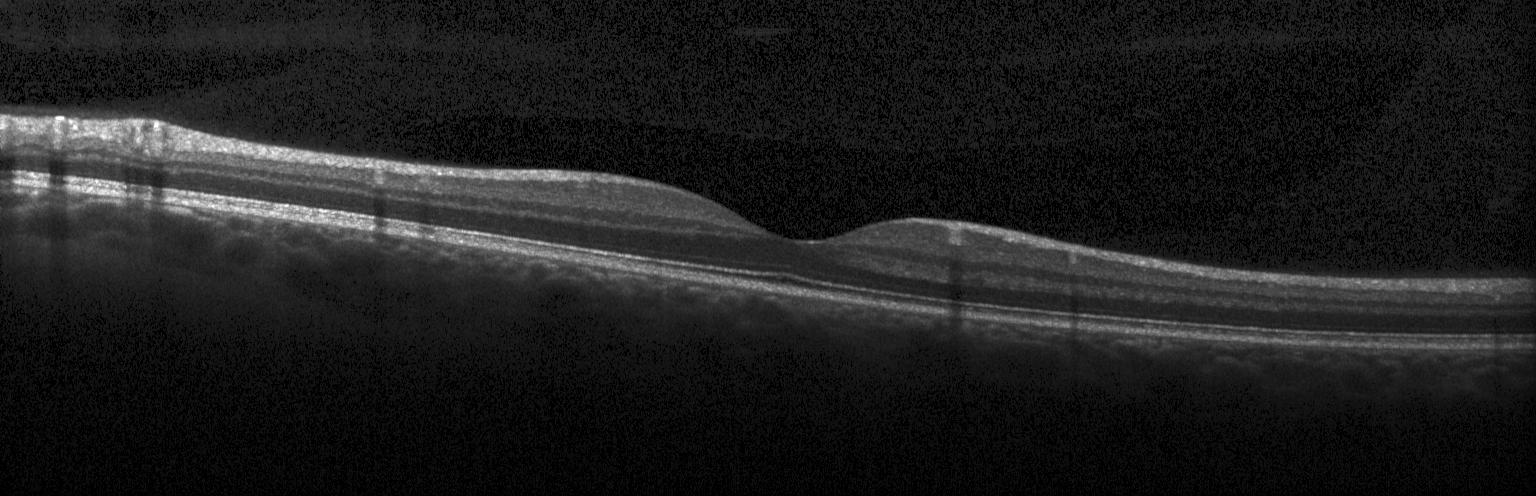
Optical coherence tomography B-scan. Finding: neither choroidal neovascularization, diabetic macular edema, nor drusen.